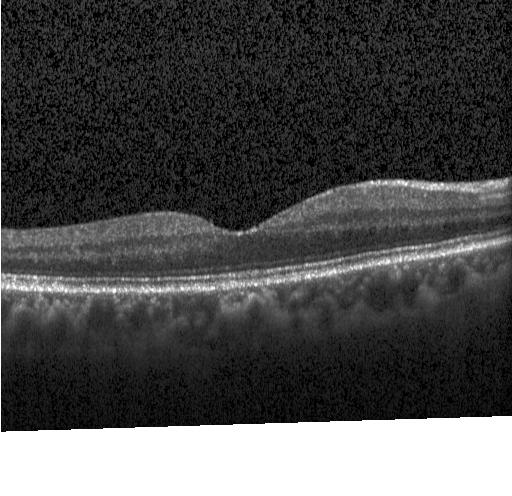 Retinal OCT cross-section; acquired on a Heidelberg Spectralis; centered on the fovea; spectral-domain OCT.
Impression: no choroidal neovascularization, no diabetic macular edema, and no drusen.